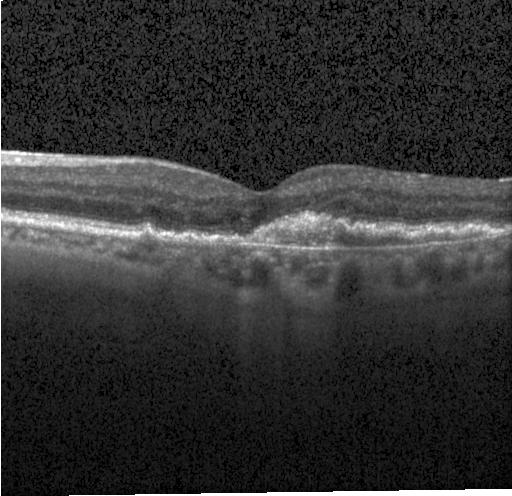 Horizontal scan through the fovea, OCT line scan. A choroidal neovascular membrane.